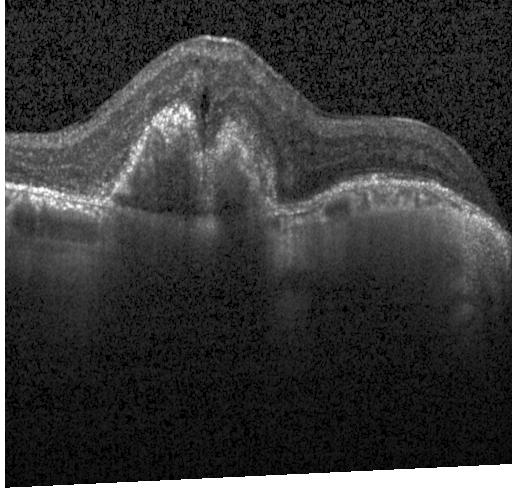 Fovea-centered, optical coherence tomography scan. Finding: a choroidal neovascular membrane.